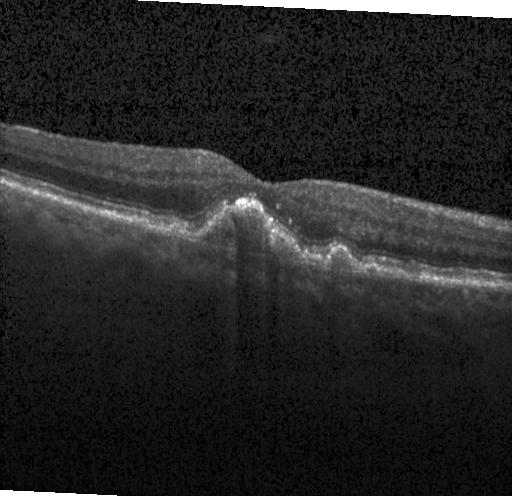 Spectral-domain optical coherence tomography, macular scan, OCT line scan, acquired on a Heidelberg Spectralis
Diagnosis: a choroidal neovascular membrane.